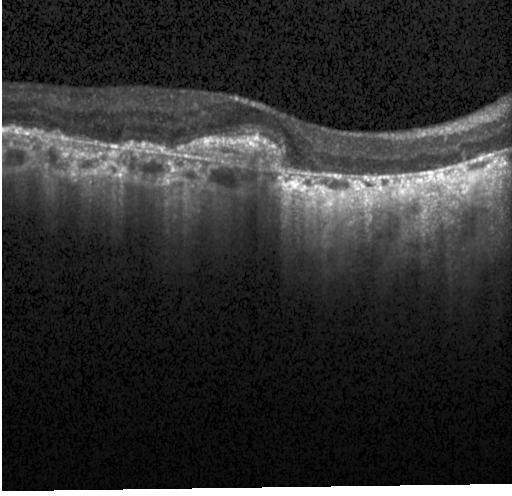

Spectral-domain OCT; optical coherence tomography B-scan
OCT finding: a choroidal neovascular membrane.